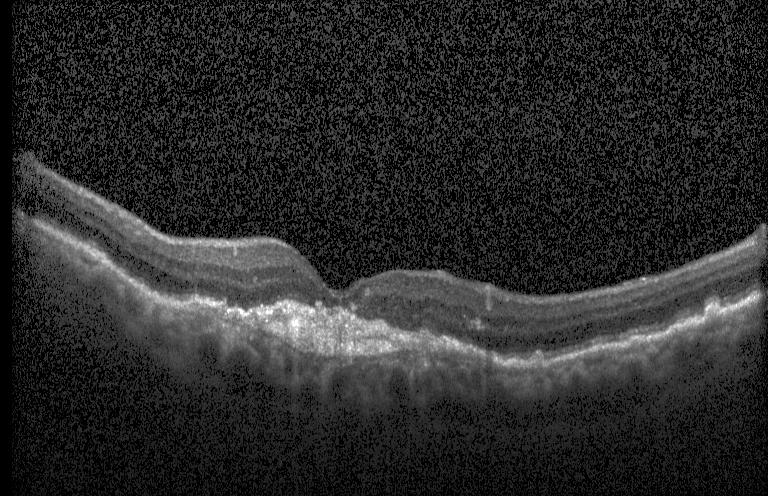 Optical coherence tomography B-scan. Spectral-domain OCT. Heidelberg Spectralis. Horizontal scan through the fovea — This B-scan demonstrates CNV.